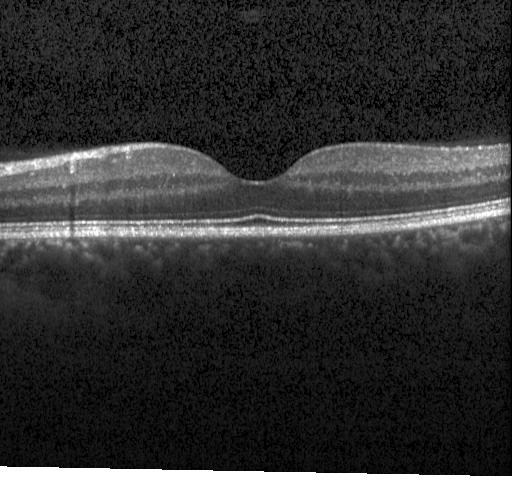

Spectral-domain OCT B-scan: no choroidal neovascularization, no diabetic macular edema, and no drusen.